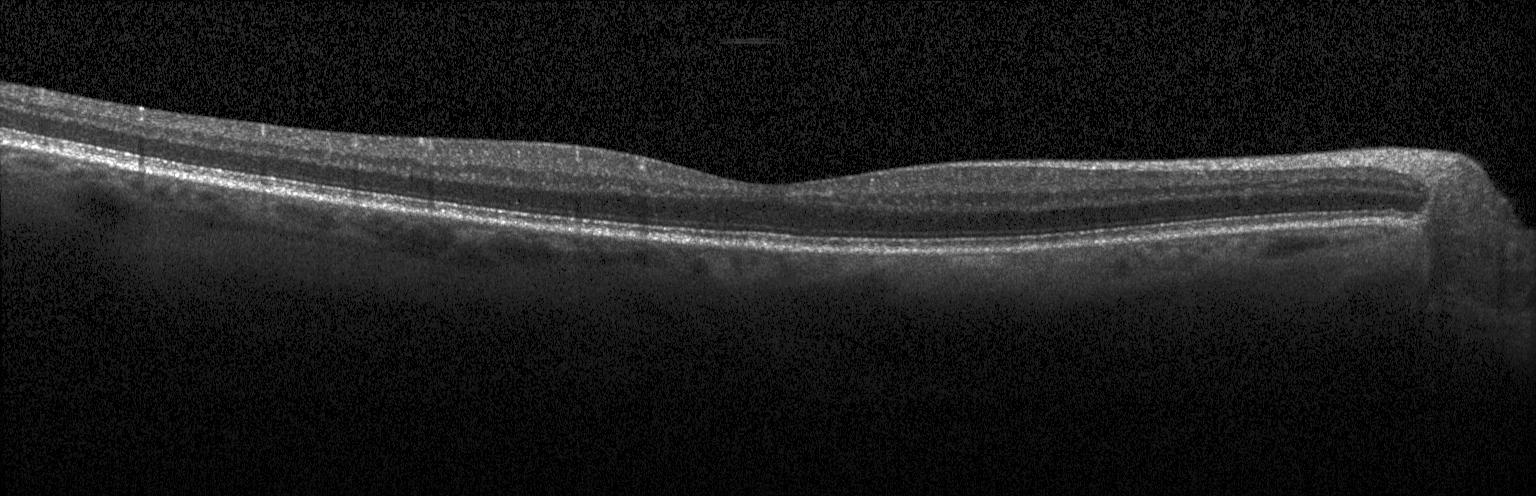 The scan shows no choroidal neovascularization, no diabetic macular edema, and no drusen.